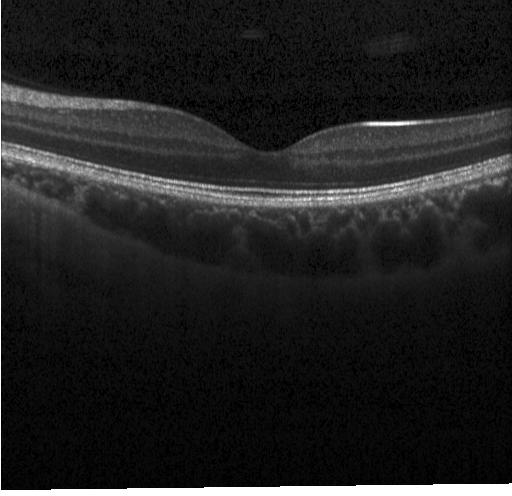
OCT B-scan. Assessment: no choroidal neovascularization, diabetic macular edema, or drusen.